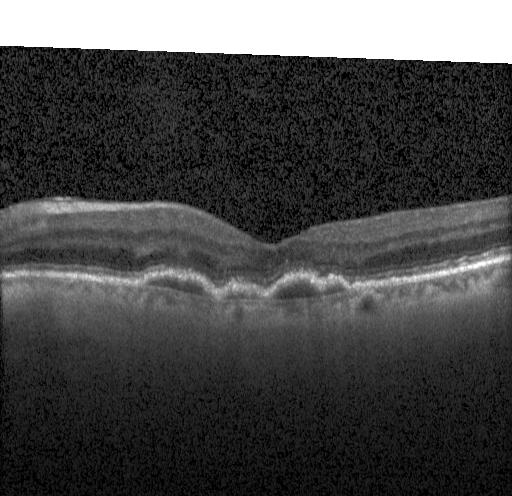

Optical coherence tomography B-scan · horizontal scan through the fovea · spectral-domain optical coherence tomography. Diagnosis: choroidal neovascularization (CNV).